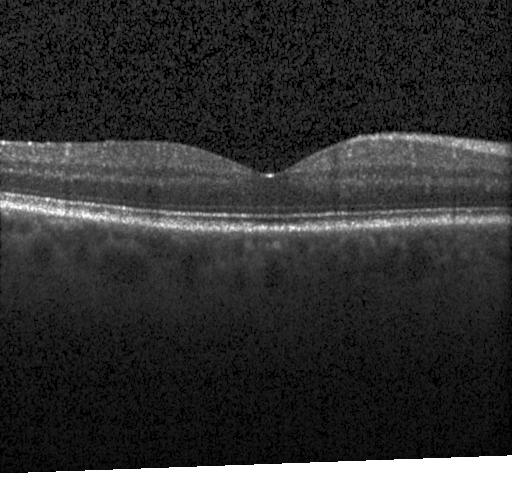

OCT line scan. Finding: neither choroidal neovascularization, diabetic macular edema, nor drusen.